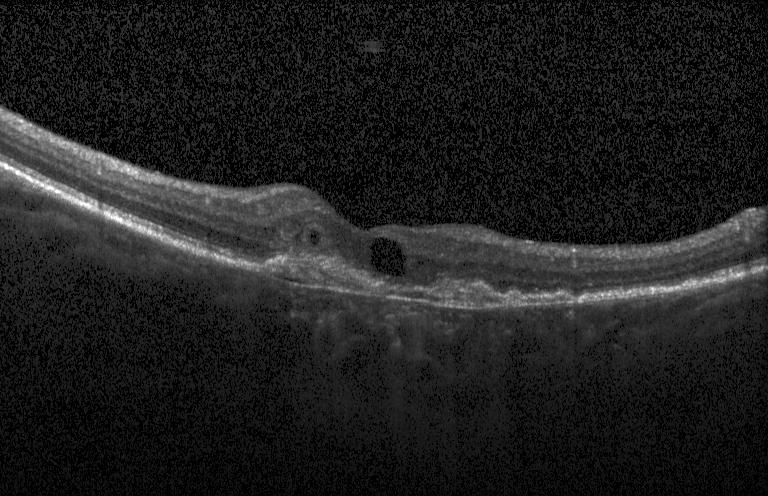 Macular OCT: a choroidal neovascular membrane.